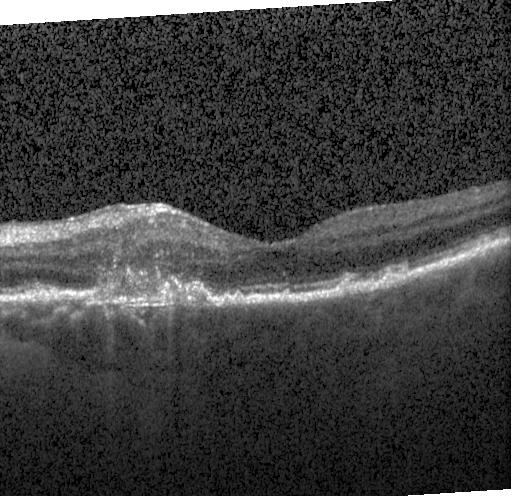

Macular scan · SD-OCT · OCT B-scan
Finding: choroidal neovascularization (CNV).